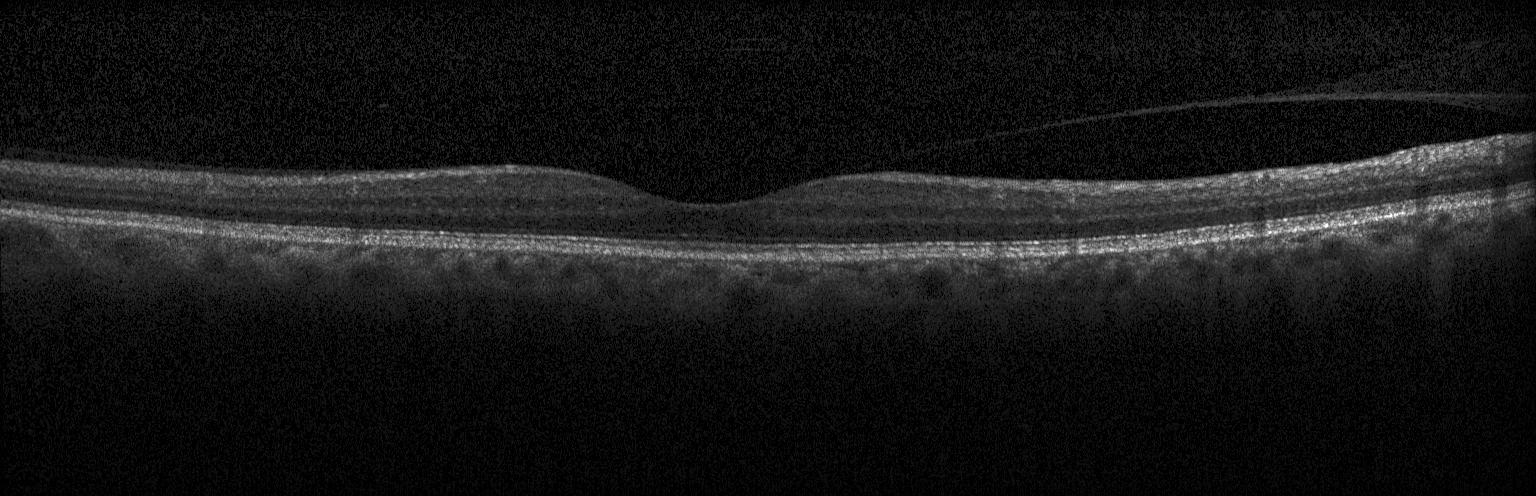 Centered on the fovea, optical coherence tomography scan
Dx: no evidence of choroidal neovascularization, diabetic macular edema, or drusen.